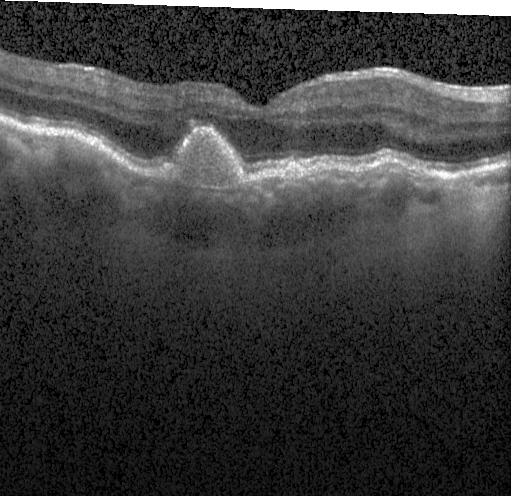

Retinal OCT cross-section, horizontal scan through the fovea.
Impression: choroidal neovascularization.